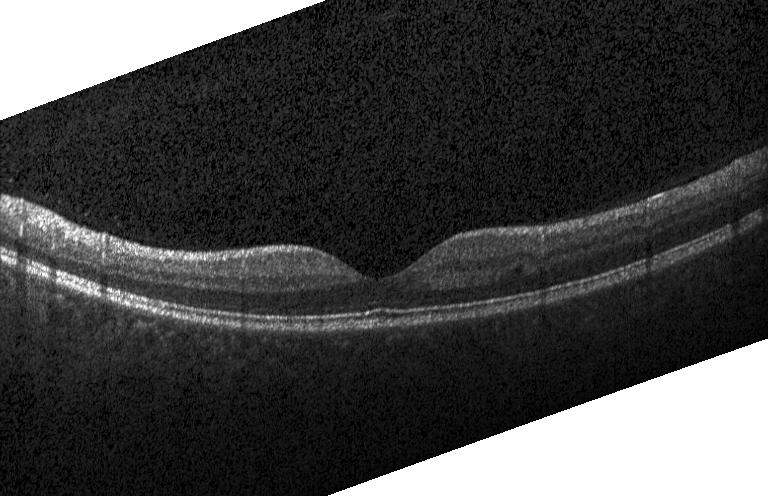 Impression: no evidence of CNV, DME, or drusen.